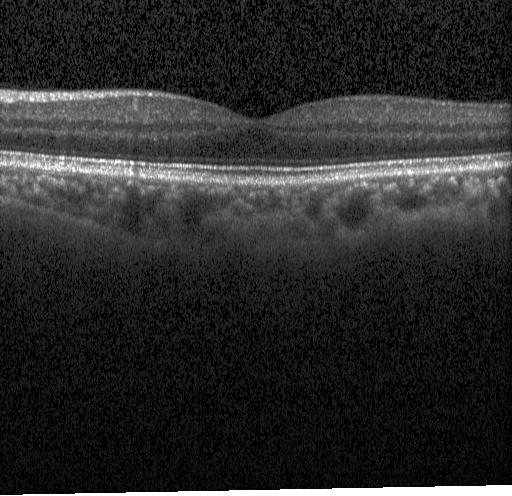 Fovea-centered. Optical coherence tomography B-scan. Spectral-domain OCT.
OCT finding: neither CNV, DME, nor drusen.